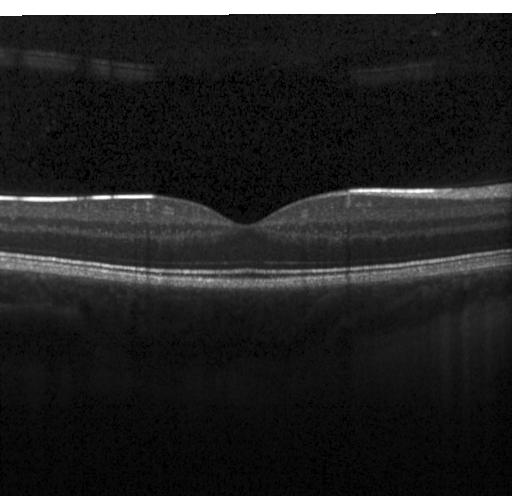

Impression: neither choroidal neovascularization, diabetic macular edema, nor drusen.